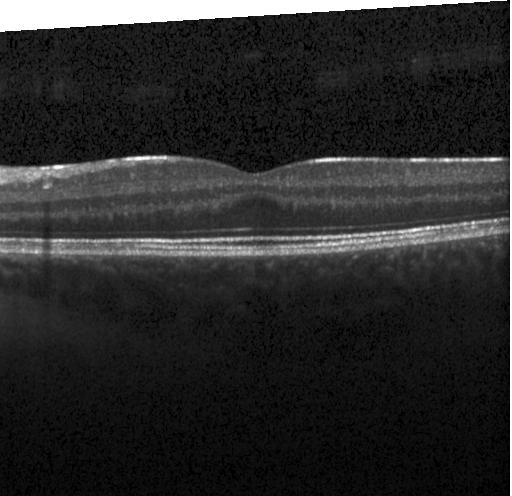

Horizontal scan through the fovea · Heidelberg Spectralis · OCT line scan · SD-OCT
Diagnosis: neither choroidal neovascularization, diabetic macular edema, nor drusen.